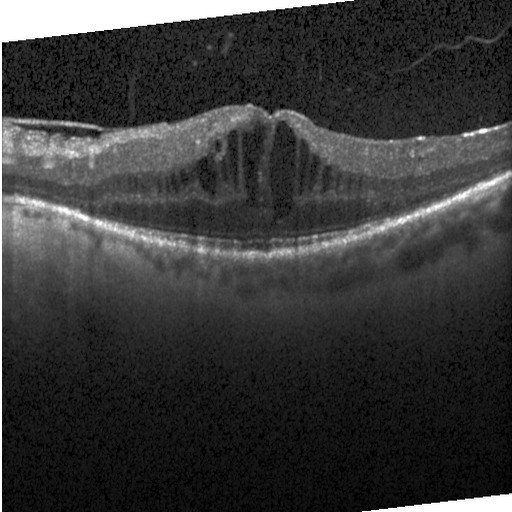
Centered on the fovea; OCT B-scan; SD-OCT; instrument: Heidelberg Spectralis — Impression: DME.